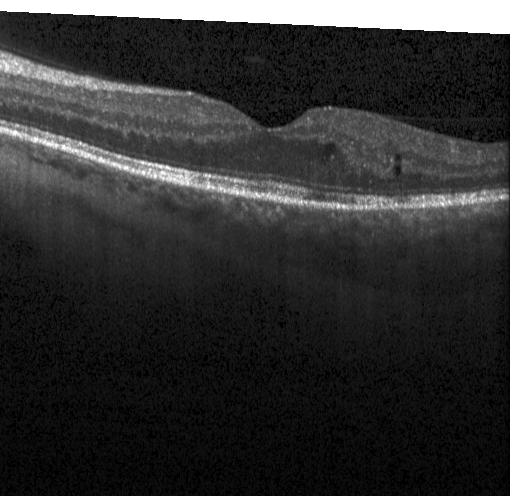

Heidelberg Spectralis OCT system, retinal OCT B-scan, SD-OCT, through the macula — The scan shows diabetic macular edema (DME).